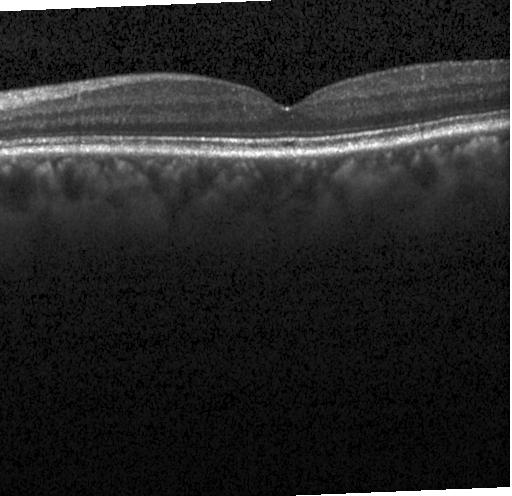 OCT B-scan. Spectral-domain OCT. Heidelberg Spectralis OCT system. The scan shows no CNV, no DME, and no drusen.